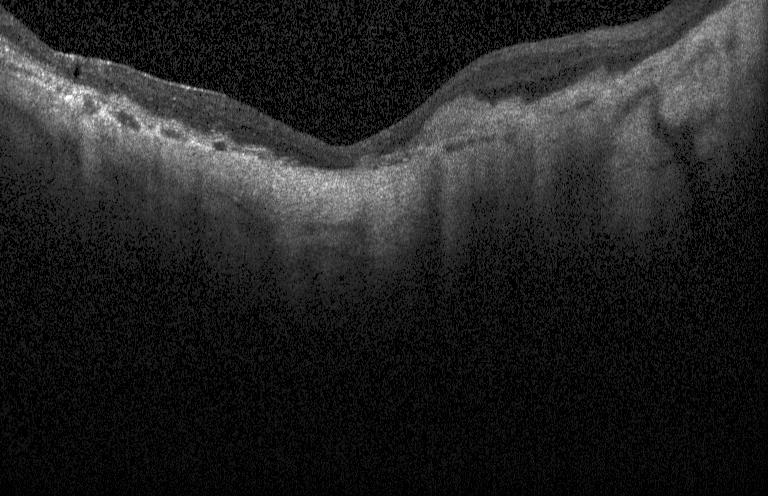 Diagnosis: choroidal neovascularization (CNV).